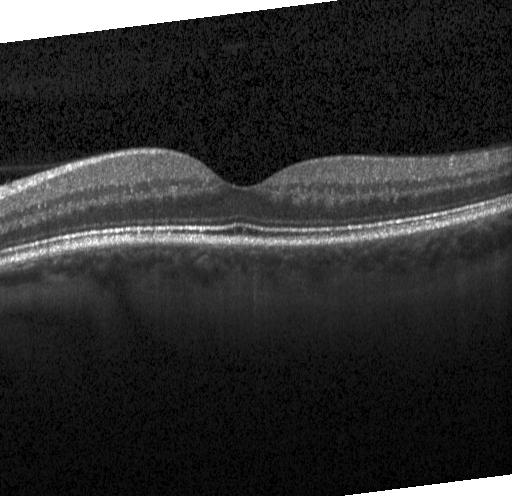

Impression: neither choroidal neovascularization, diabetic macular edema, nor drusen.